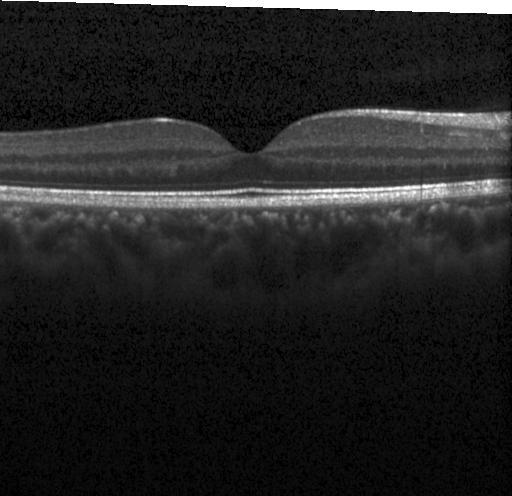
Optical coherence tomography scan · Heidelberg Spectralis — Assessment: no evidence of CNV, DME, or drusen.